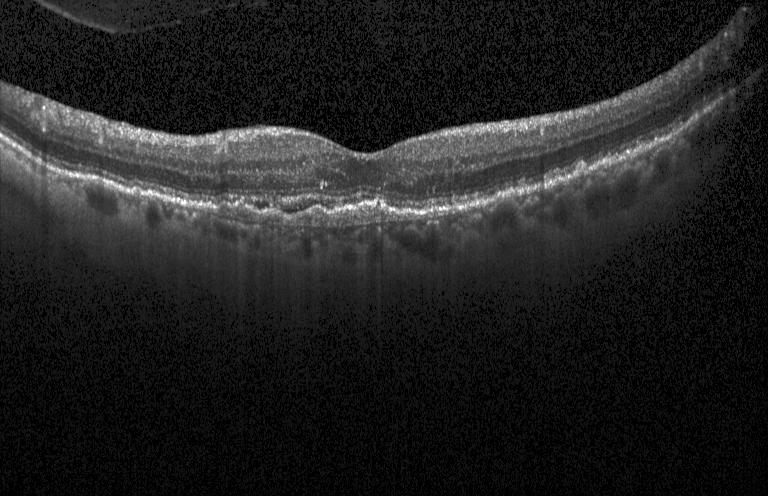 Retinal OCT B-scan, spectral-domain OCT — Macular OCT: a choroidal neovascular membrane.